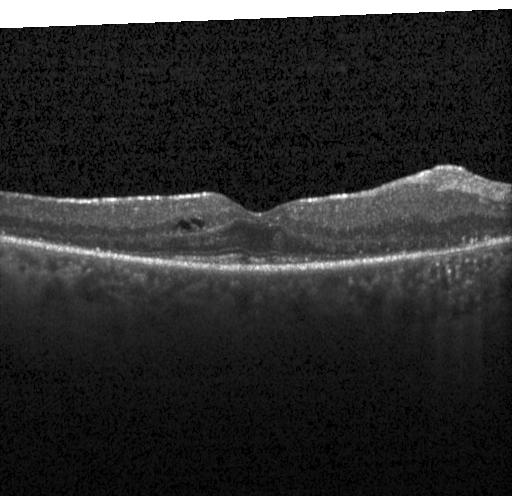

Spectral-domain OCT. Retinal OCT cross-section
Impression: diabetic macular edema.